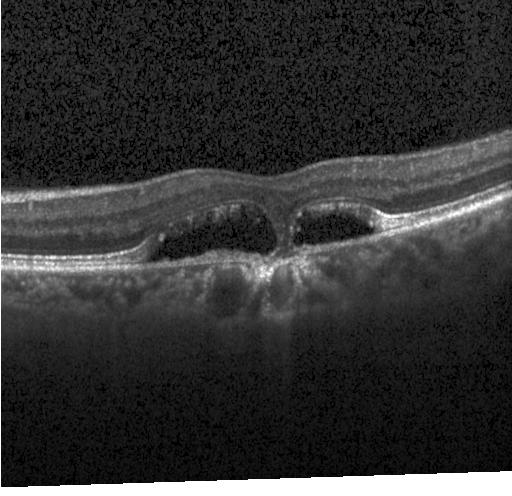 Diagnosis: a choroidal neovascular membrane.